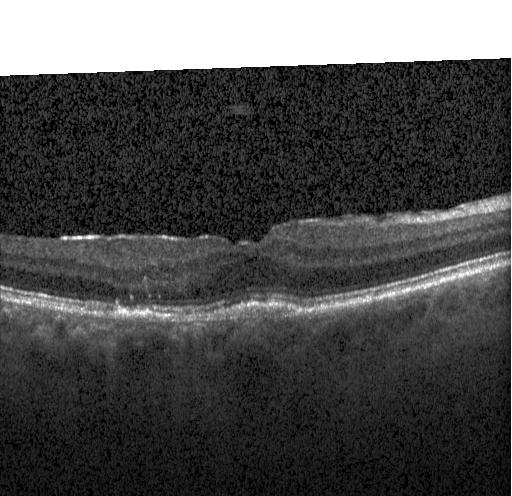
OCT scan showing a choroidal neovascular membrane.